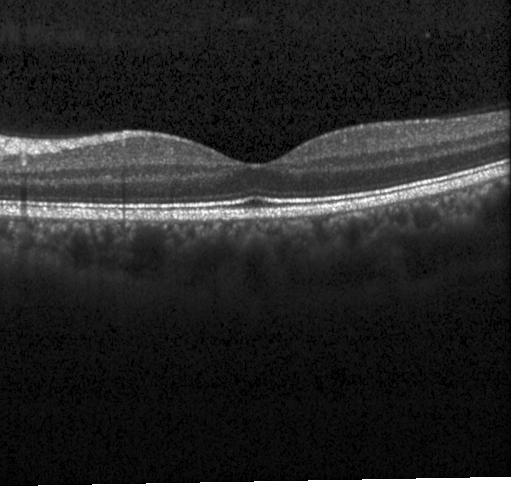

Optical coherence tomography scan — Assessment: neither CNV, DME, nor drusen.